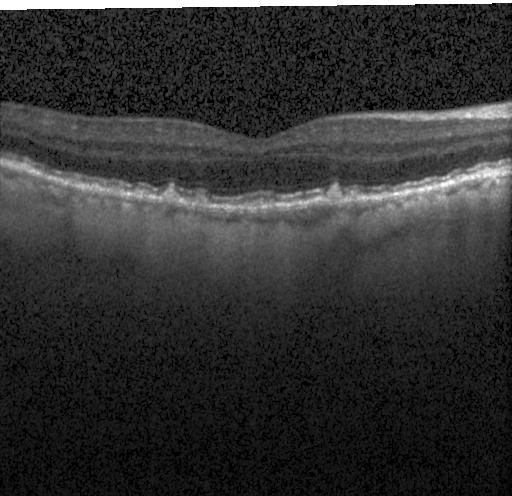

Retinal OCT B-scan · Heidelberg Spectralis · macular scan · spectral-domain OCT — Diagnosis: sub-RPE drusenoid deposits.